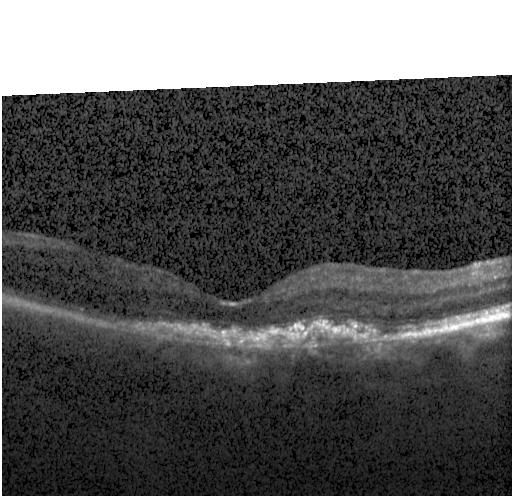
OCT finding: choroidal neovascularization.